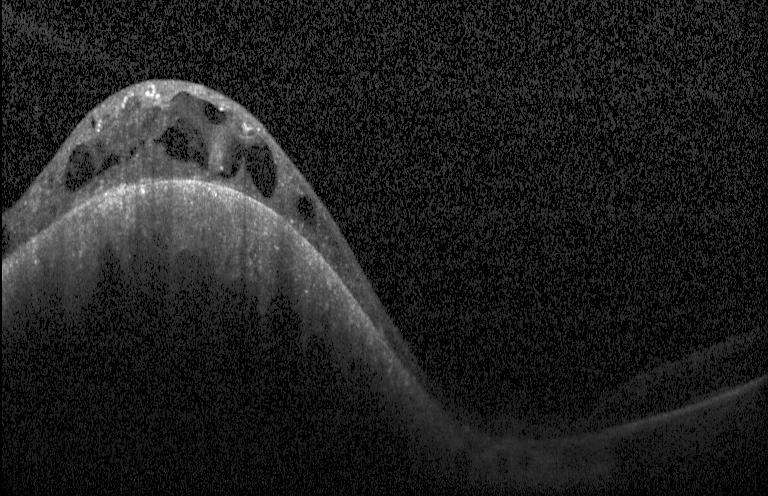
Heidelberg Spectralis; optical coherence tomography B-scan. Diagnosis: diabetic macular edema (DME).